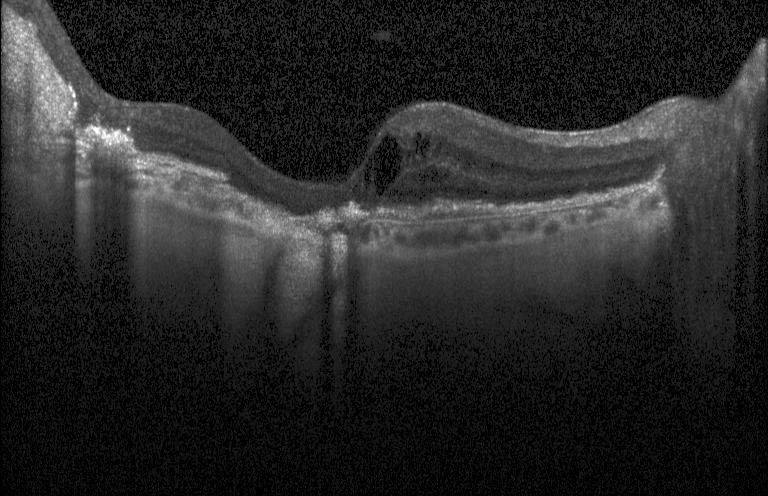 Finding: CNV.